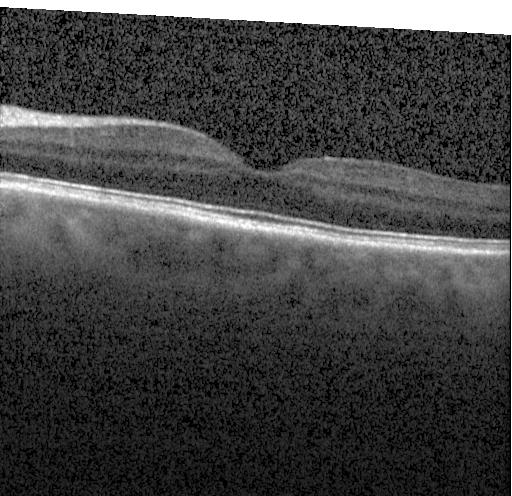 Centered on the fovea; Heidelberg Spectralis OCT system; OCT B-scan.
The scan shows no choroidal neovascularization, no diabetic macular edema, and no drusen.